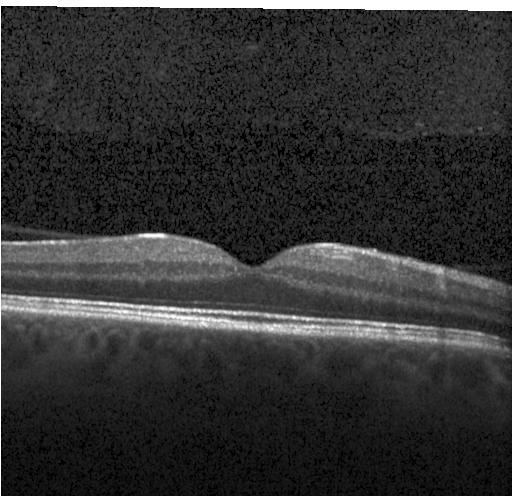

Spectral-domain OCT, macular scan, optical coherence tomography scan — Diagnosis: no choroidal neovascularization, no diabetic macular edema, and no drusen.